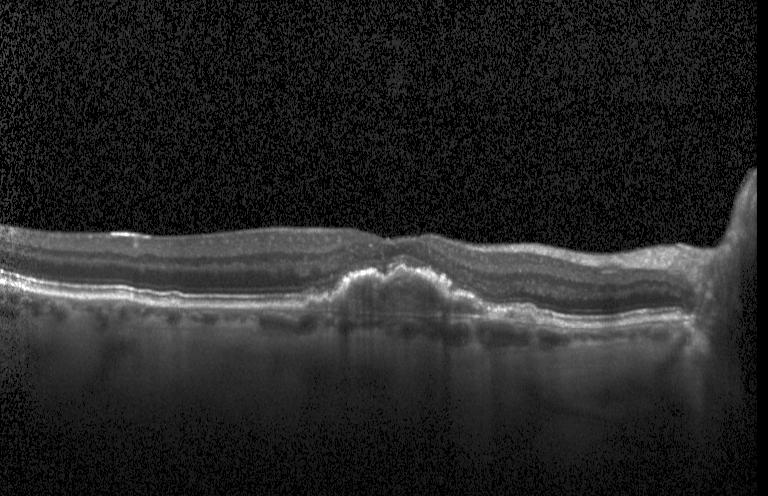
Optical coherence tomography B-scan. Macular scan
Impression: a choroidal neovascular membrane.